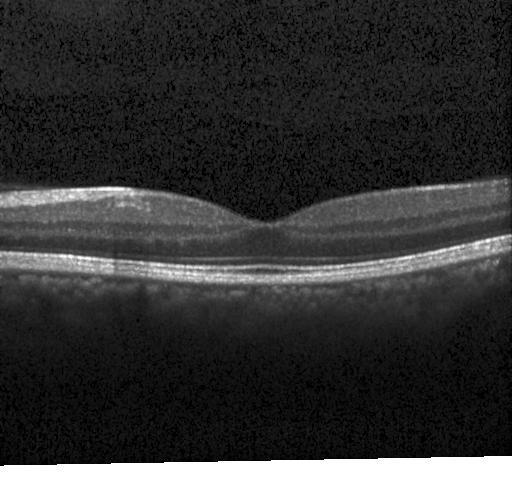
SD-OCT · acquired on a Heidelberg Spectralis · OCT line scan — This B-scan demonstrates no evidence of choroidal neovascularization, diabetic macular edema, or drusen.